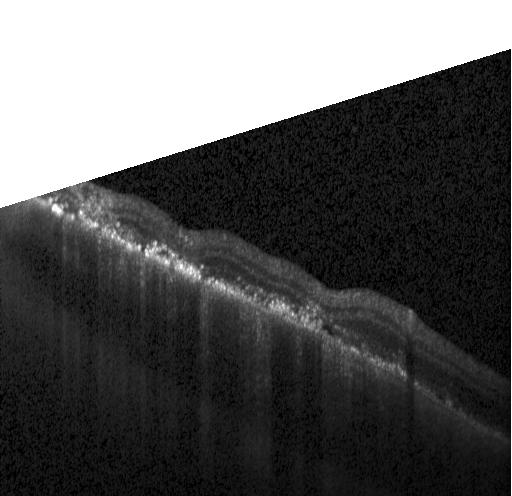 Impression: choroidal neovascularization (CNV).